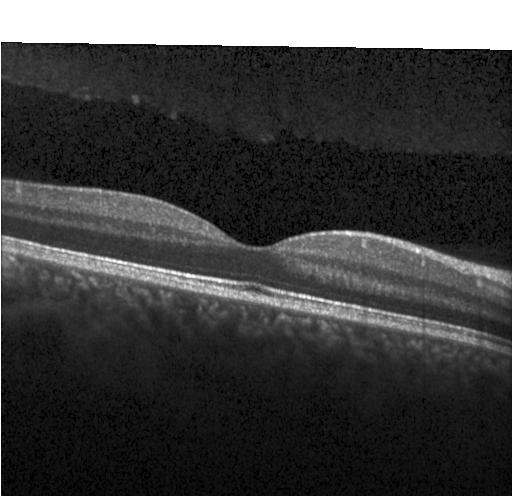 Instrument: Heidelberg Spectralis. OCT B-scan.
This B-scan demonstrates no choroidal neovascularization, diabetic macular edema, or drusen.